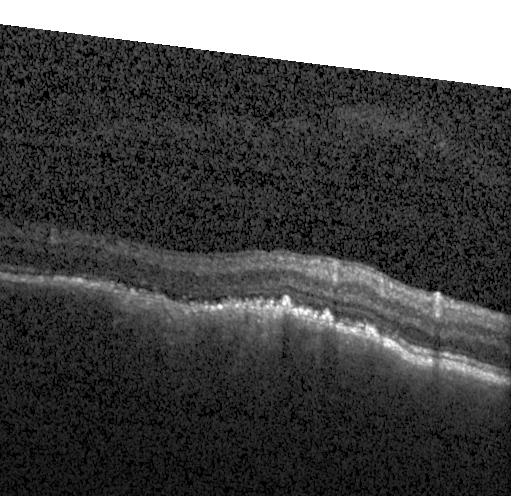 Retinal OCT cross-section, through the macula, acquired on a Heidelberg Spectralis, spectral-domain OCT
Finding: a choroidal neovascular membrane.